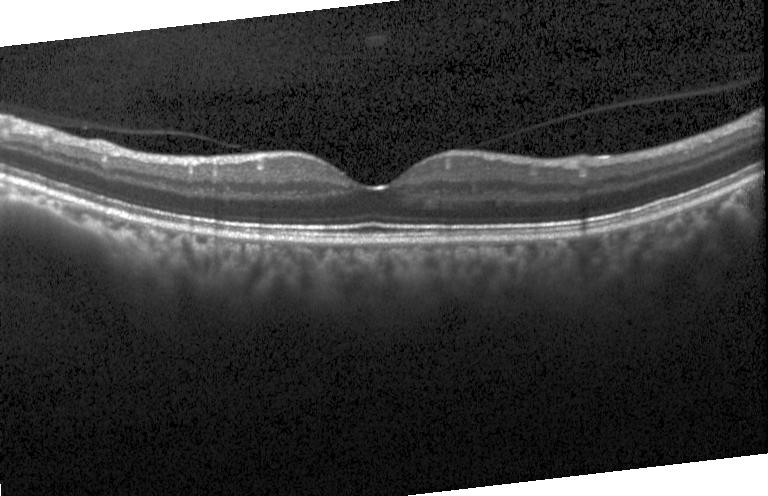

Diagnosis: no choroidal neovascularization, no diabetic macular edema, and no drusen.